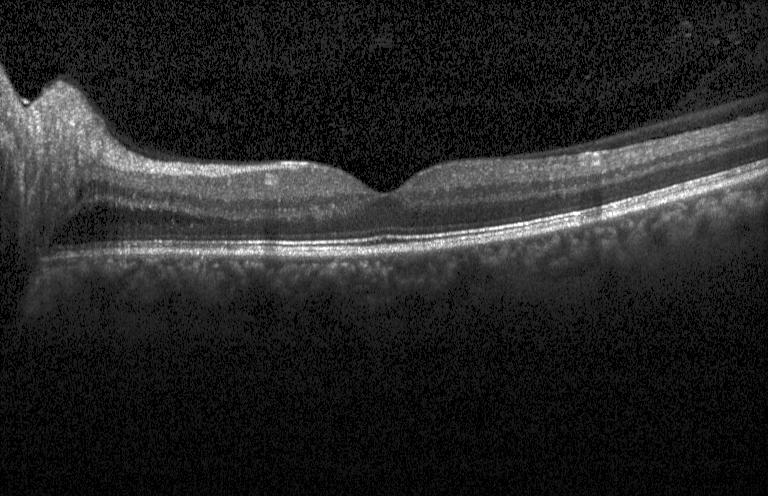 Retinal OCT cross-section.
No CNV, DME, or drusen.